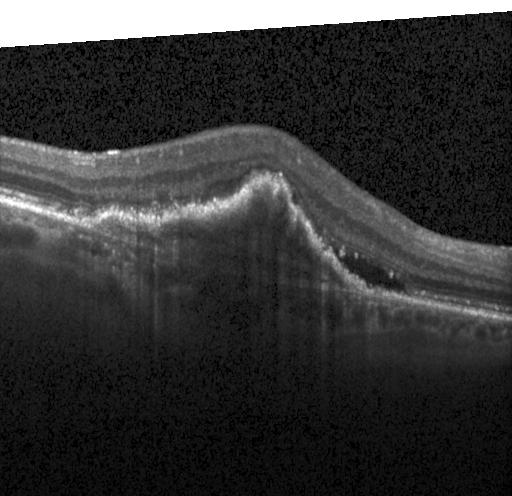

Macular scan · optical coherence tomography scan · spectral-domain optical coherence tomography — Impression: choroidal neovascularization.